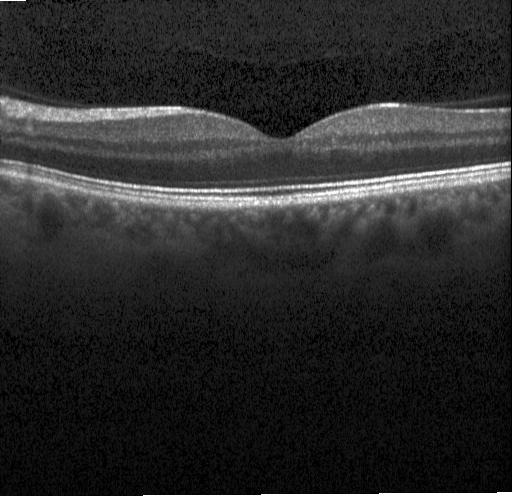

Acquired on a Heidelberg Spectralis; spectral-domain optical coherence tomography; retinal OCT B-scan
The scan shows no CNV, no DME, and no drusen.